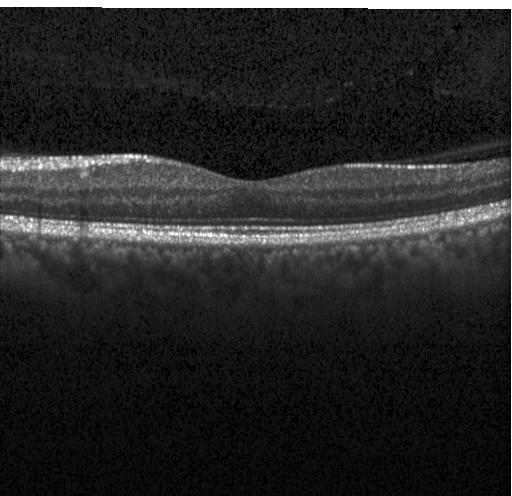 OCT line scan. Horizontal scan through the fovea. Heidelberg Spectralis OCT system. Spectral-domain OCT.
Dx: no choroidal neovascularization, diabetic macular edema, or drusen.